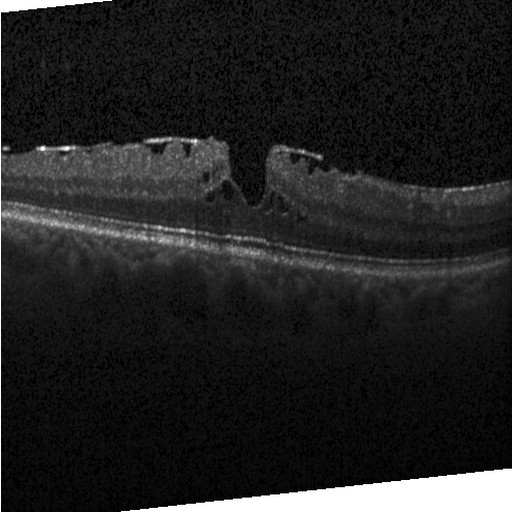

Optical coherence tomography B-scan. Finding: diabetic macular edema.